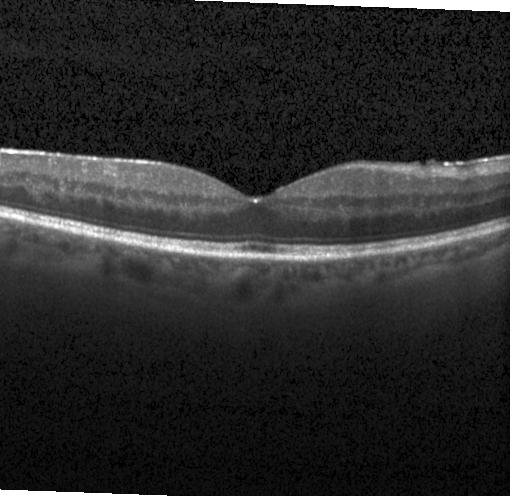
Spectral-domain OCT; acquired on a Heidelberg Spectralis; optical coherence tomography scan.
Finding: no choroidal neovascularization, no diabetic macular edema, and no drusen.